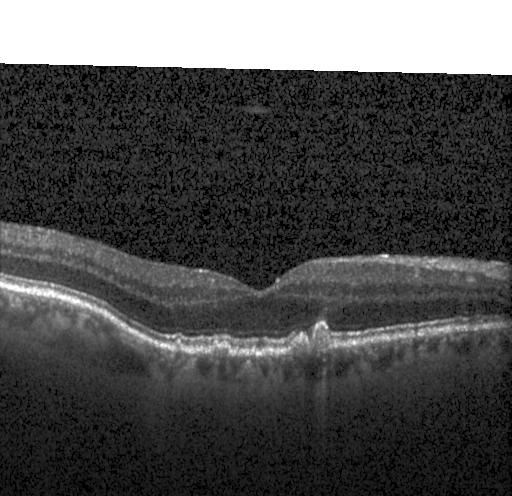
Instrument: Heidelberg Spectralis. Retinal OCT B-scan. Spectral-domain OCT. Assessment: multiple drusen.